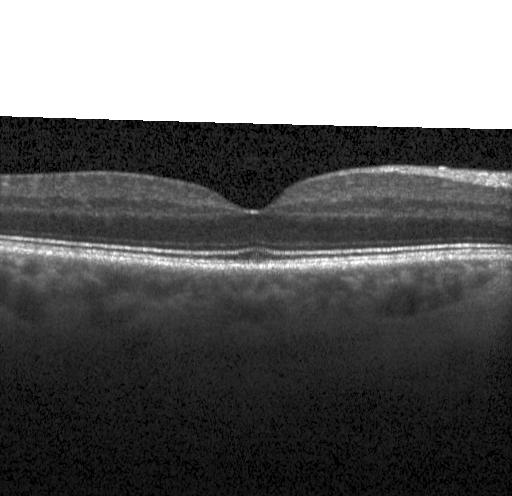 No CNV, DME, or drusen.